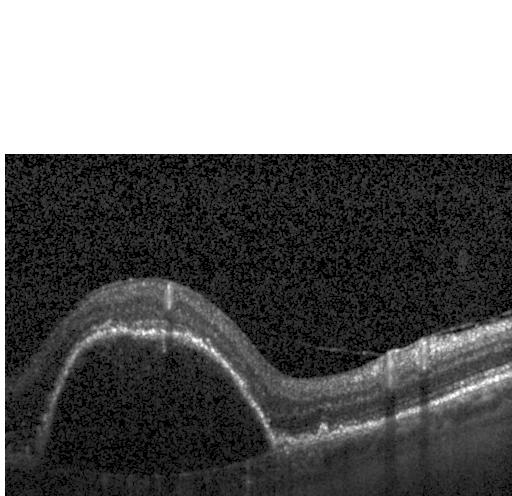
The scan shows choroidal neovascularization (CNV).